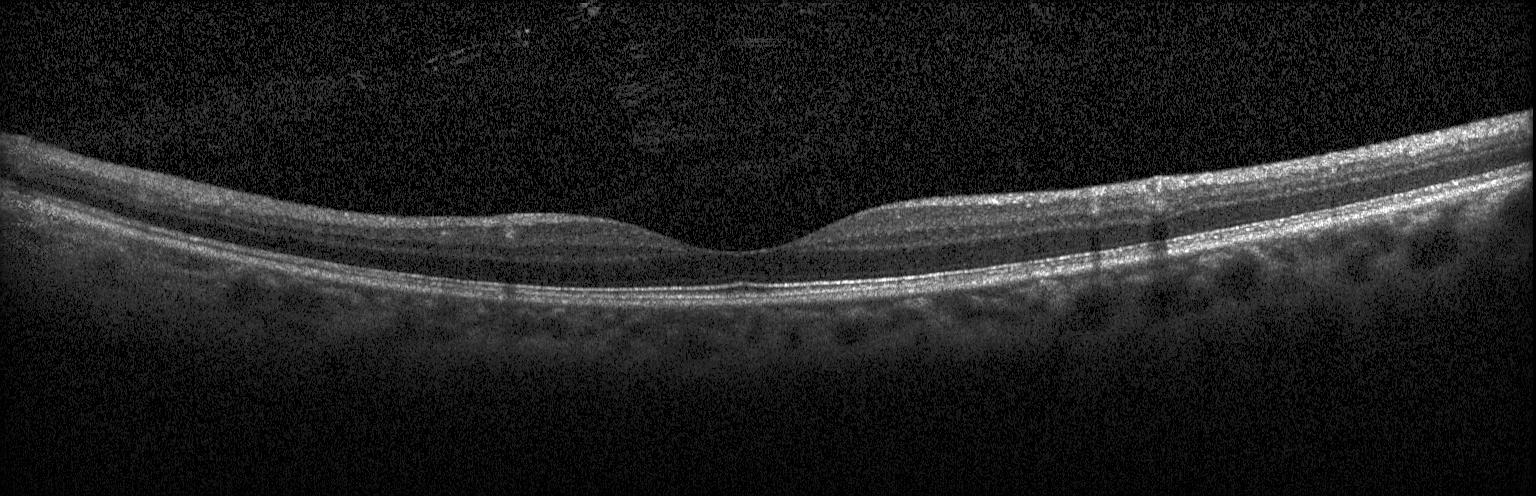

Macular OCT demonstrating no evidence of CNV, DME, or drusen.